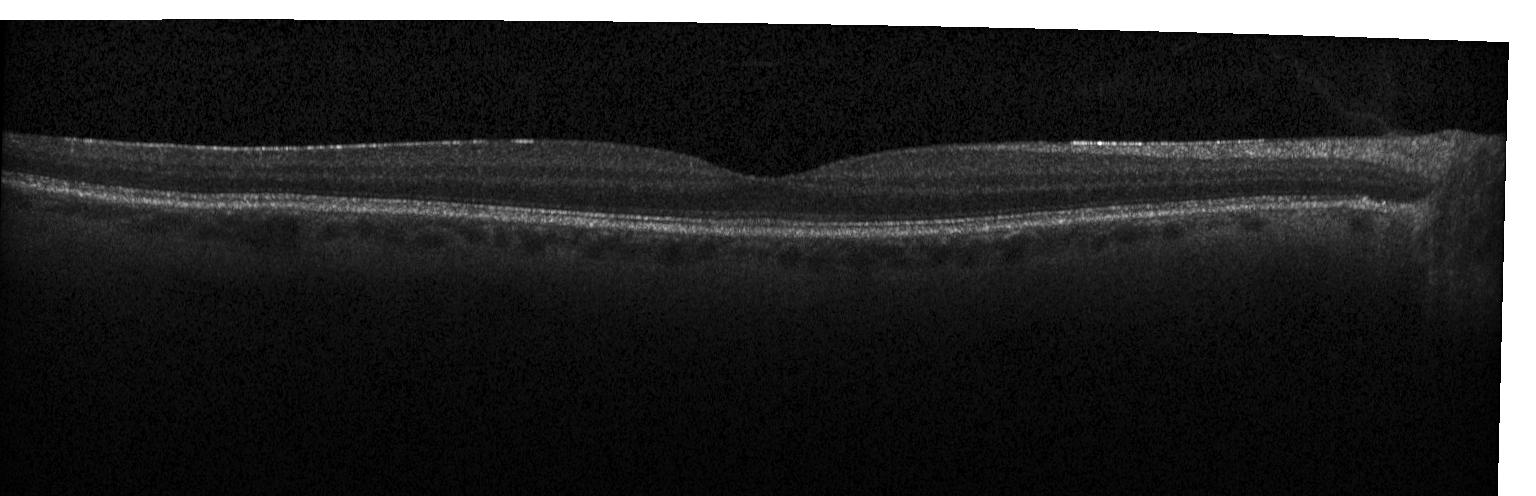

Acquired on a Heidelberg Spectralis. SD-OCT. Macular scan. OCT B-scan — Finding: no CNV, no DME, and no drusen.